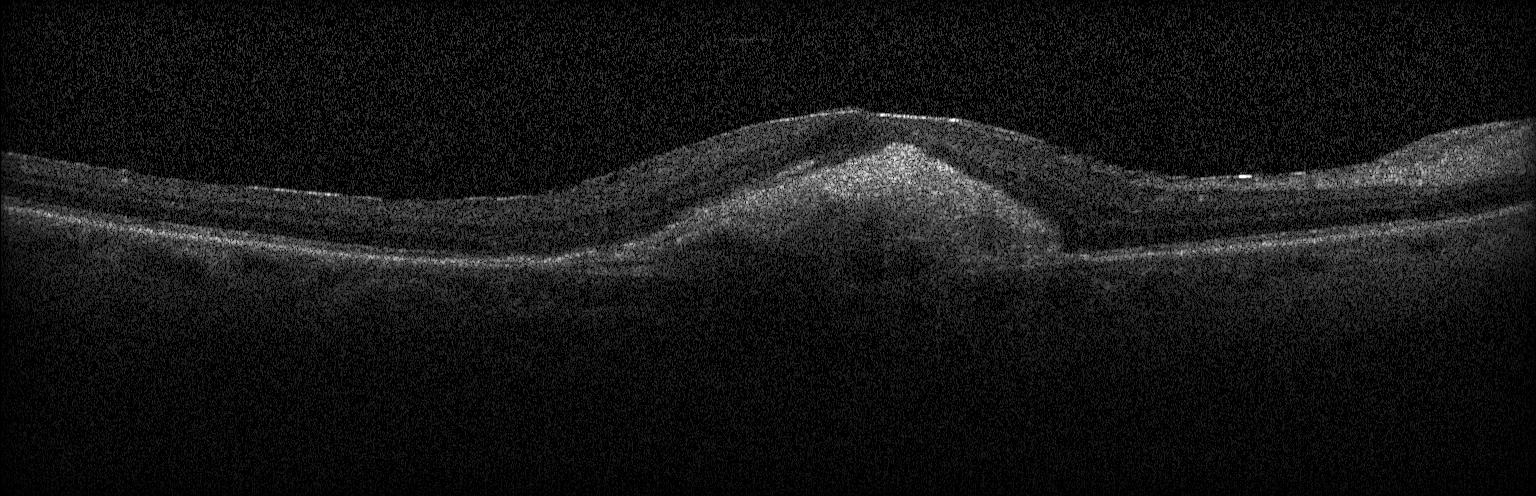

Macular OCT demonstrating CNV.